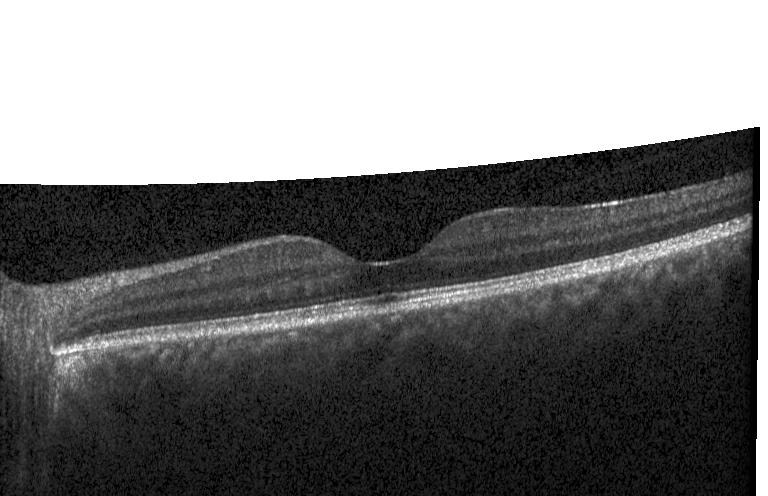
Fovea-centered; spectral-domain OCT; retinal OCT cross-section; Heidelberg Spectralis OCT system — Finding: neither CNV, DME, nor drusen.